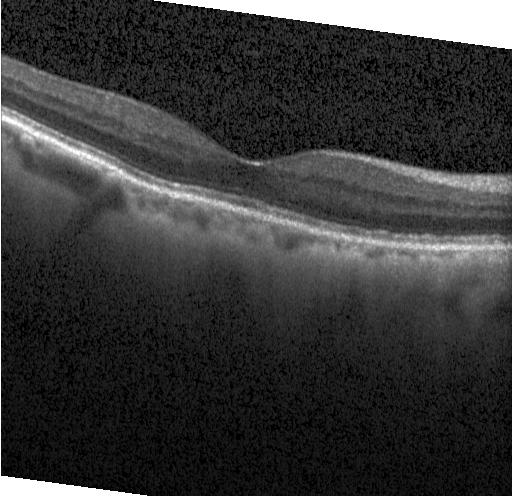 SD-OCT · OCT line scan. Impression: no choroidal neovascularization, diabetic macular edema, or drusen.